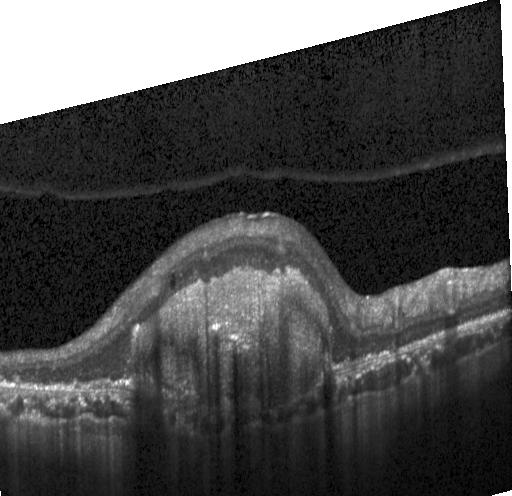 OCT B-scan; spectral-domain optical coherence tomography — Finding: a choroidal neovascular membrane.